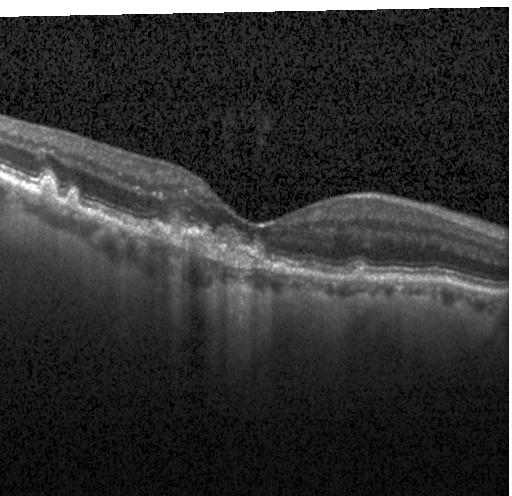 Optical coherence tomography B-scan. This B-scan demonstrates choroidal neovascularization (CNV).